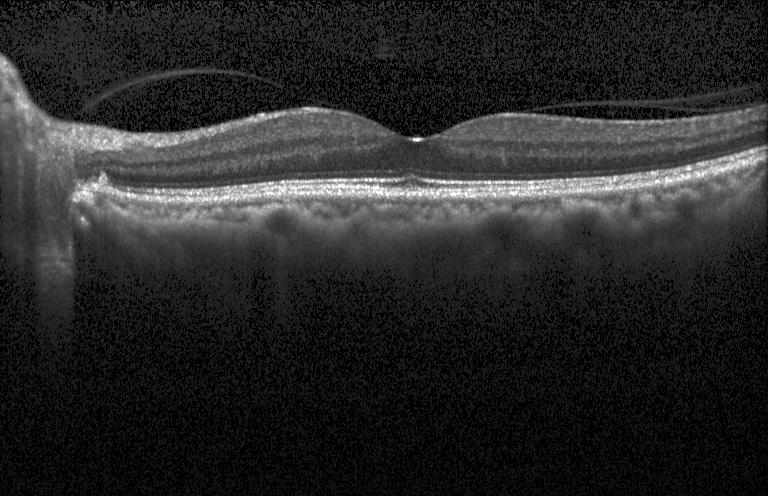
Retinal OCT B-scan. Heidelberg Spectralis. Horizontal scan through the fovea — Assessment: no choroidal neovascularization, no diabetic macular edema, and no drusen.